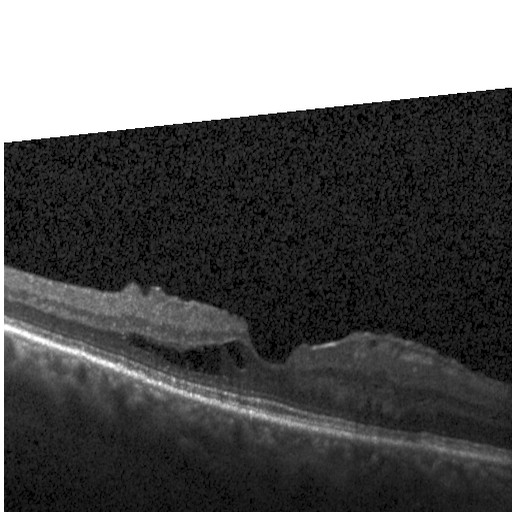 OCT B-scan; SD-OCT. OCT finding: DME.